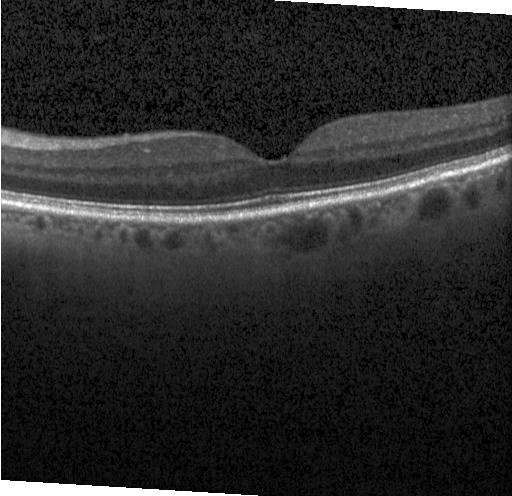
Centered on the fovea · Heidelberg Spectralis · OCT line scan
This B-scan demonstrates no choroidal neovascularization, diabetic macular edema, or drusen.